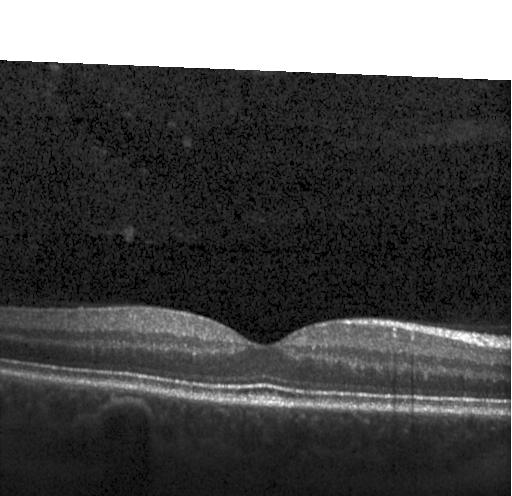
OCT scan showing no choroidal neovascularization, no diabetic macular edema, and no drusen.